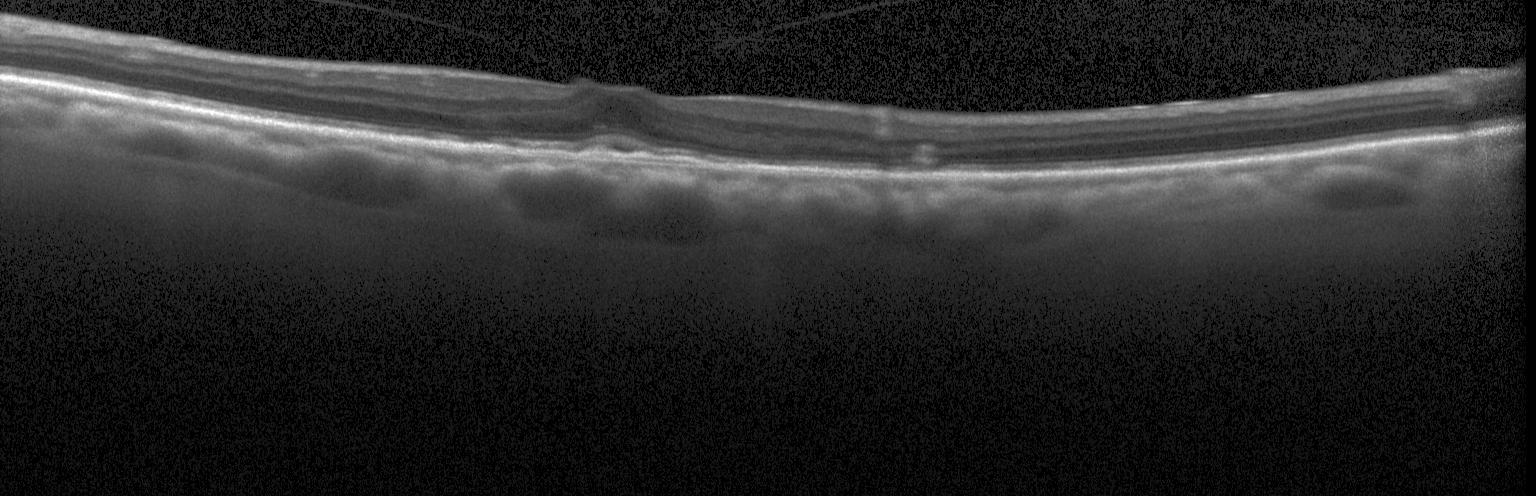

SD-OCT · OCT line scan
A choroidal neovascular membrane.